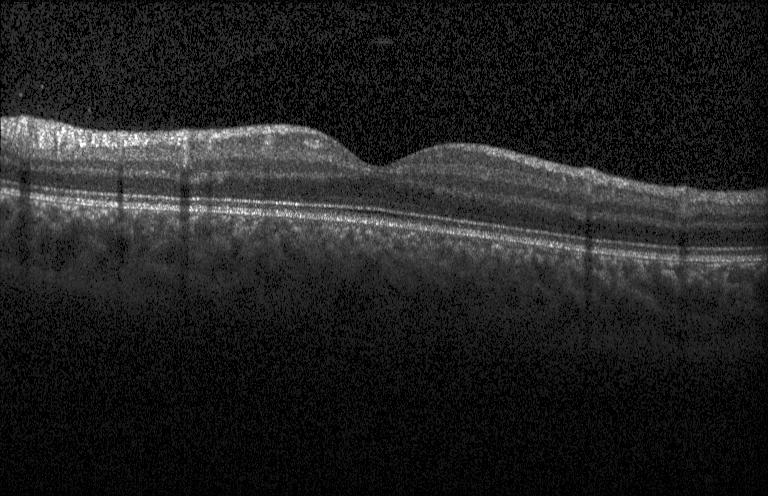 Optical coherence tomography scan; Heidelberg Spectralis OCT system; spectral-domain optical coherence tomography; horizontal scan through the fovea. Impression: no evidence of CNV, DME, or drusen.